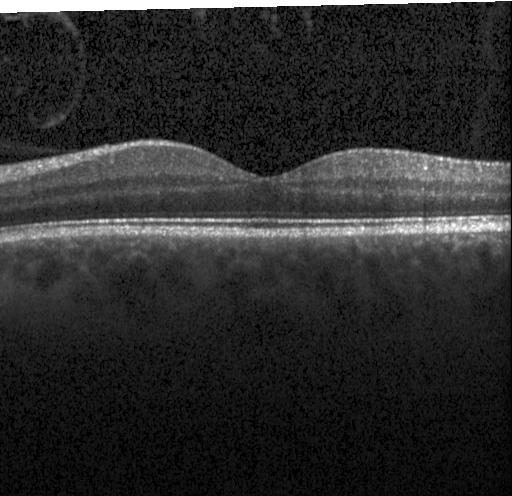

Dx: neither choroidal neovascularization, diabetic macular edema, nor drusen.